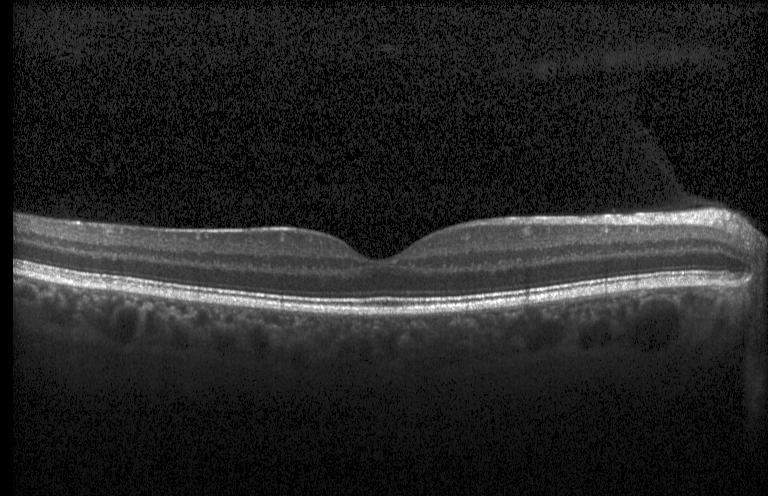
Fovea-centered, OCT B-scan, SD-OCT, Heidelberg Spectralis OCT system
The scan shows no evidence of CNV, DME, or drusen.